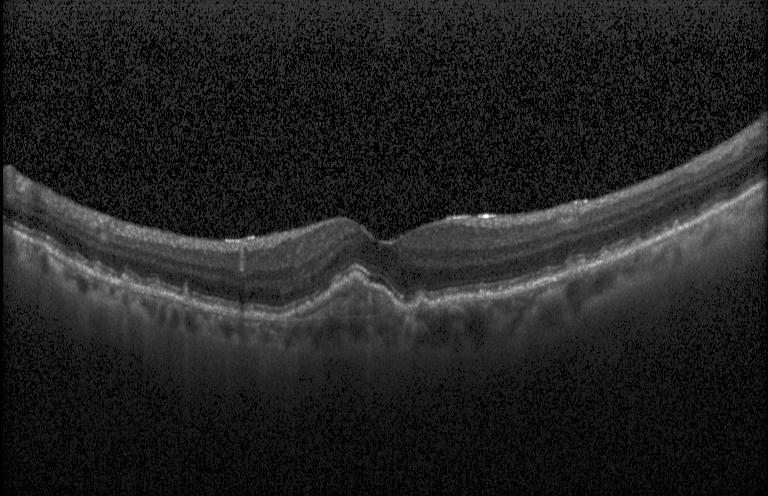 Diagnosis: a choroidal neovascular membrane.